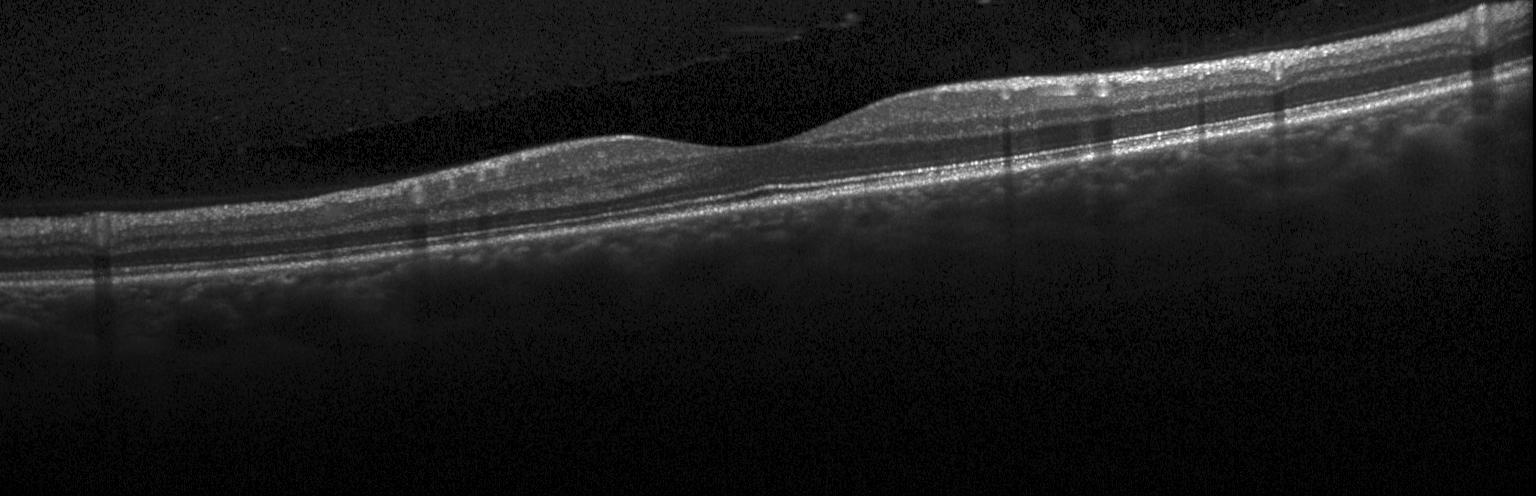
Optical coherence tomography B-scan. Spectral-domain OCT. Horizontal scan through the fovea. Heidelberg Spectralis OCT system.
Impression: no choroidal neovascularization, diabetic macular edema, or drusen.